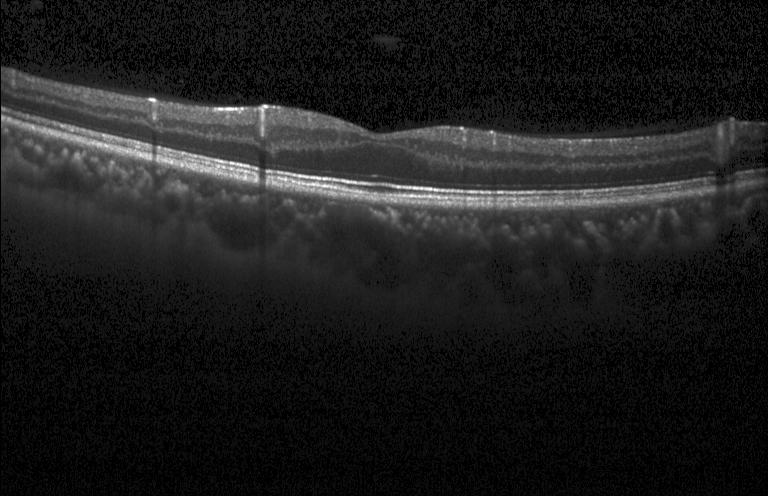
Assessment: no choroidal neovascularization, no diabetic macular edema, and no drusen.